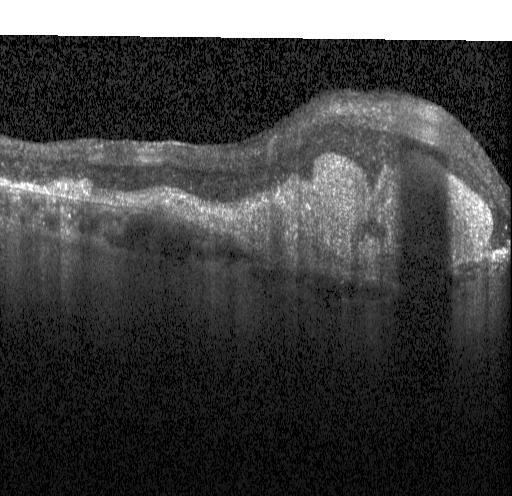 Impression: CNV.